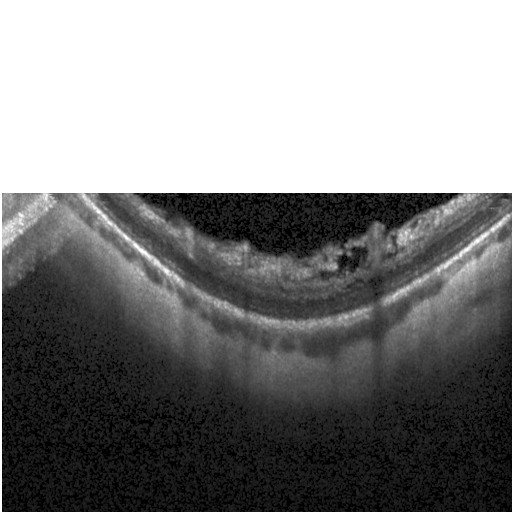 Dx: diabetic macular edema (DME).